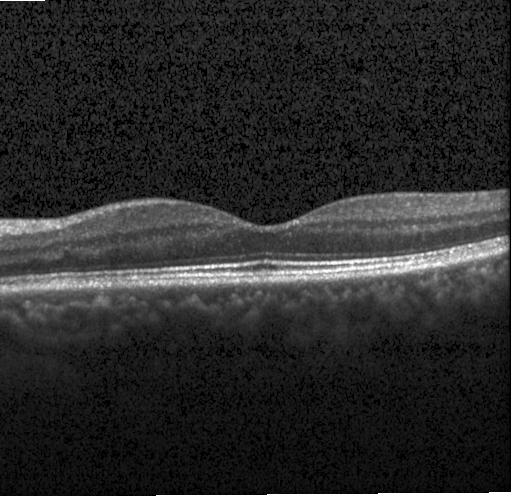

Assessment: neither choroidal neovascularization, diabetic macular edema, nor drusen.